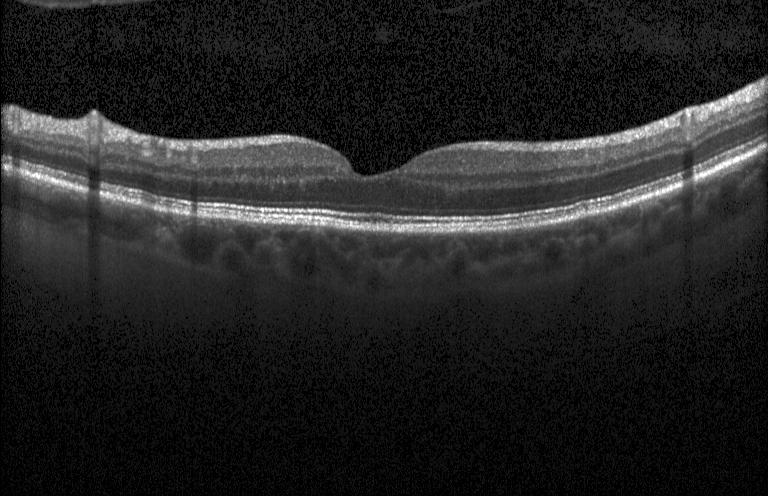
OCT line scan, through the macula. Impression: no evidence of CNV, DME, or drusen.